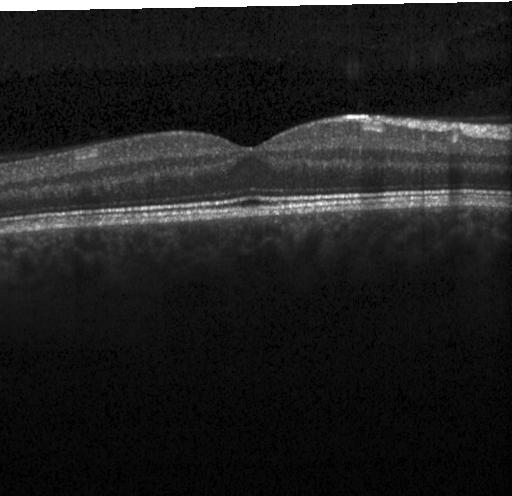 Heidelberg Spectralis, spectral-domain OCT, retinal OCT cross-section, centered on the fovea
Impression: no evidence of choroidal neovascularization, diabetic macular edema, or drusen.